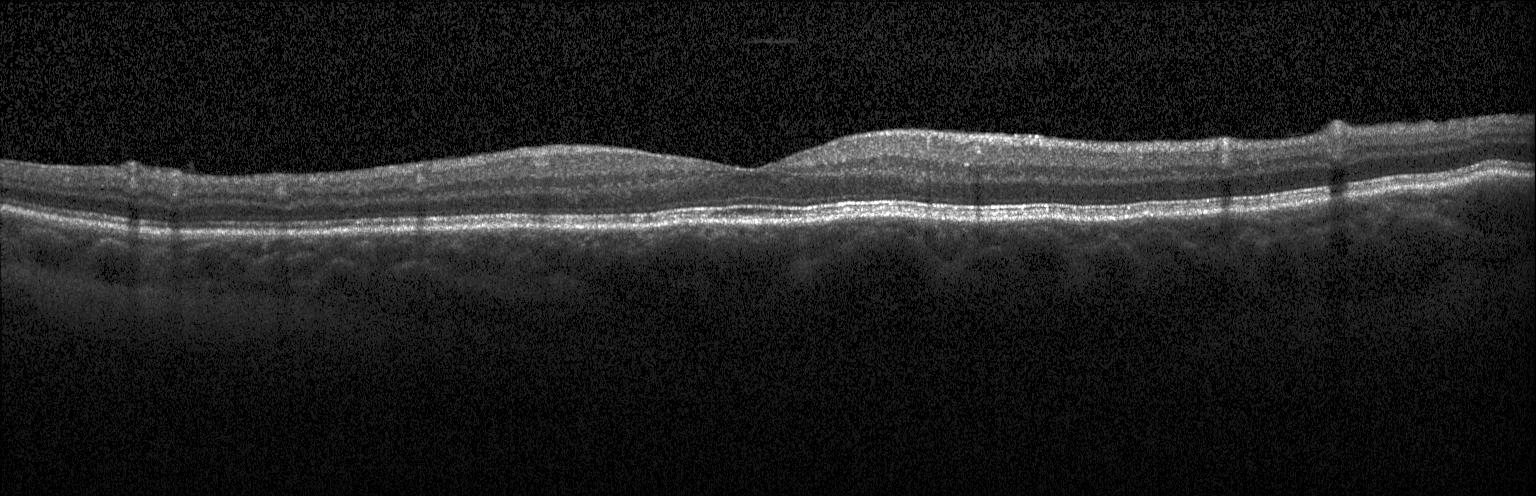

OCT finding: no CNV, DME, or drusen.